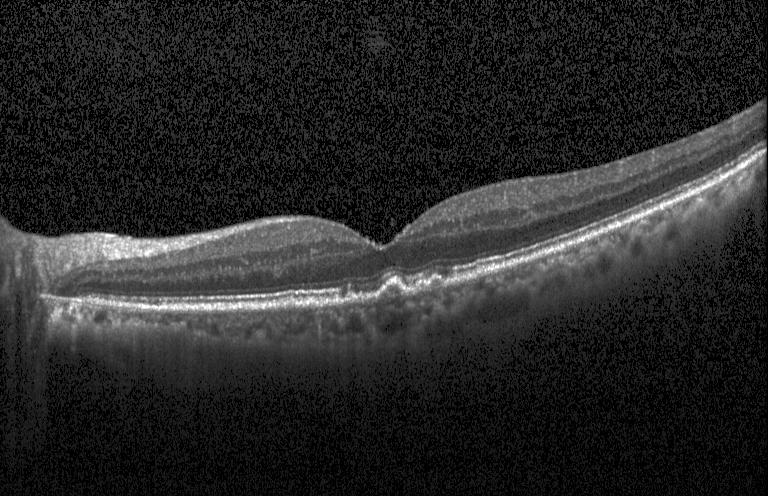 OCT line scan; centered on the fovea.
Macular OCT: multiple drusen.